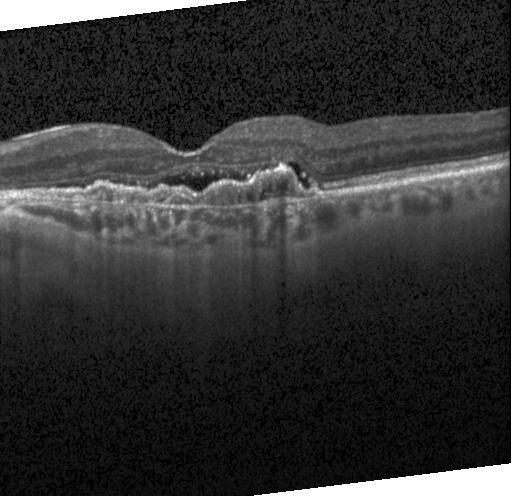 Retinal OCT B-scan · acquired on a Heidelberg Spectralis
Impression: choroidal neovascularization.